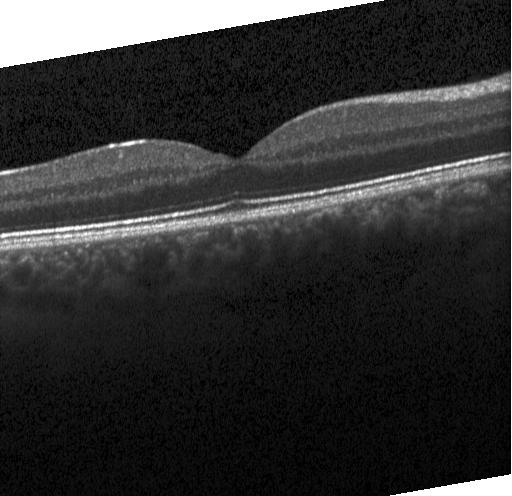

Spectral-domain OCT · optical coherence tomography B-scan. Finding: no choroidal neovascularization, no diabetic macular edema, and no drusen.